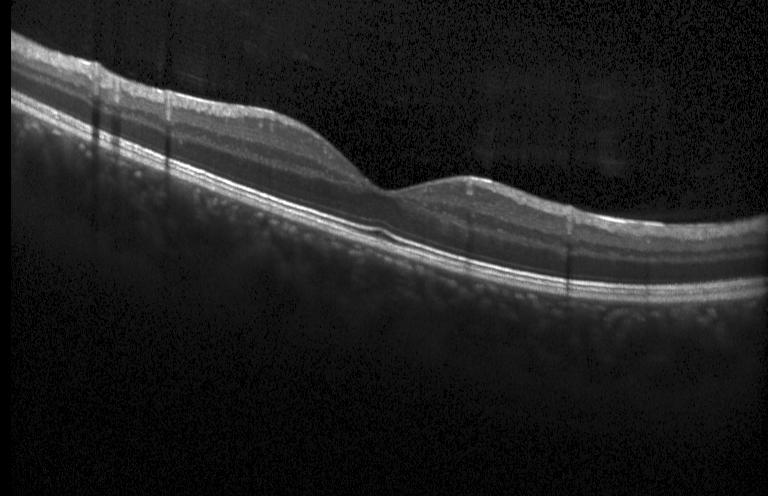 Optical coherence tomography scan. Spectral-domain OCT. Through the macula
Impression: no choroidal neovascularization, no diabetic macular edema, and no drusen.